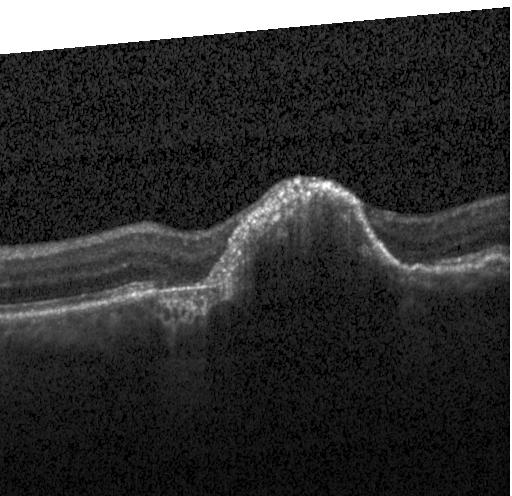

Fovea-centered, OCT B-scan, spectral-domain OCT, acquired on a Heidelberg Spectralis — Diagnosis: CNV.